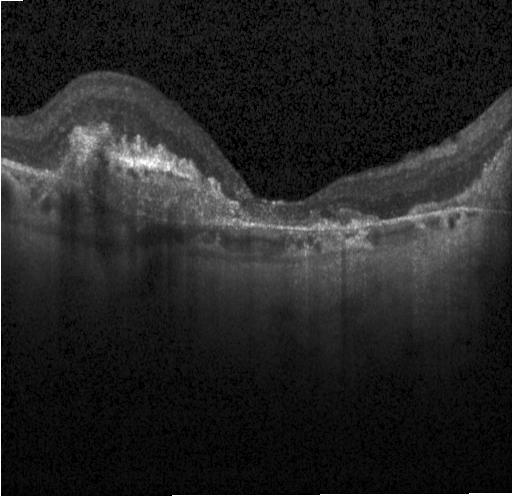

Spectral-domain OCT; centered on the fovea; Heidelberg Spectralis; optical coherence tomography scan
Finding: choroidal neovascularization.